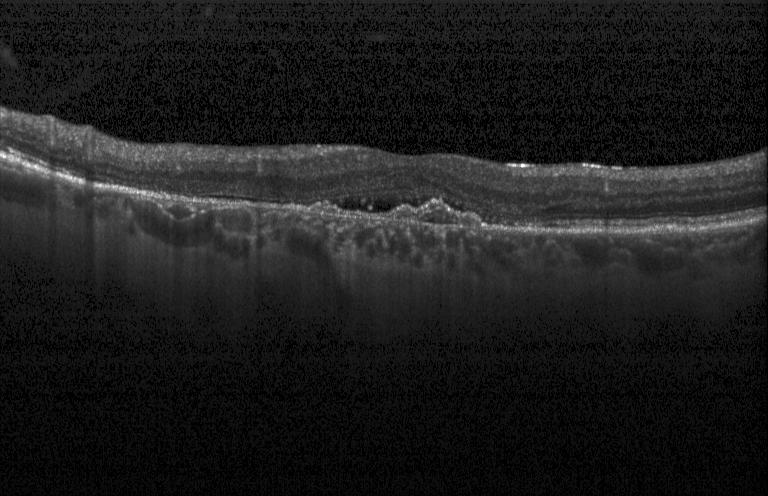 Through the macula, SD-OCT, OCT B-scan, instrument: Heidelberg Spectralis.
Dx: choroidal neovascularization (CNV).